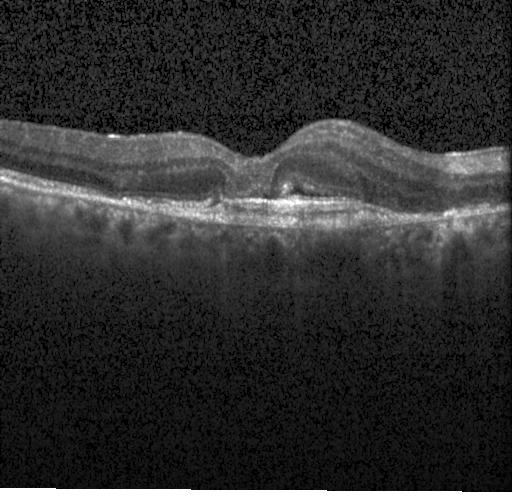
Diagnosis: choroidal neovascularization.